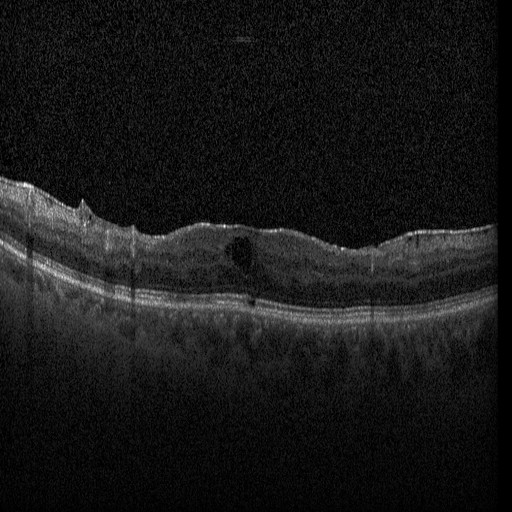
Retinal OCT cross-section showing diabetic macular edema (DME).